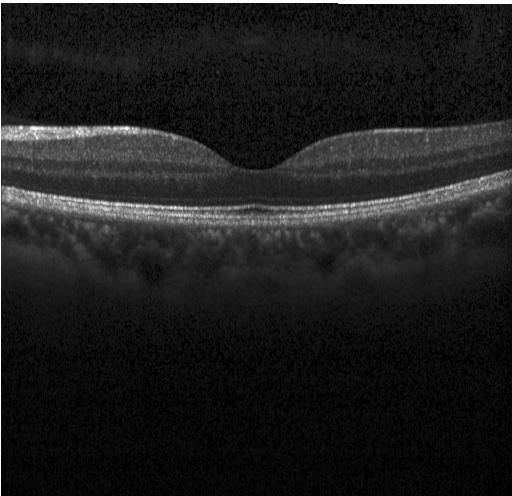

Optical coherence tomography scan; centered on the fovea; Heidelberg Spectralis
OCT finding: no CNV, no DME, and no drusen.